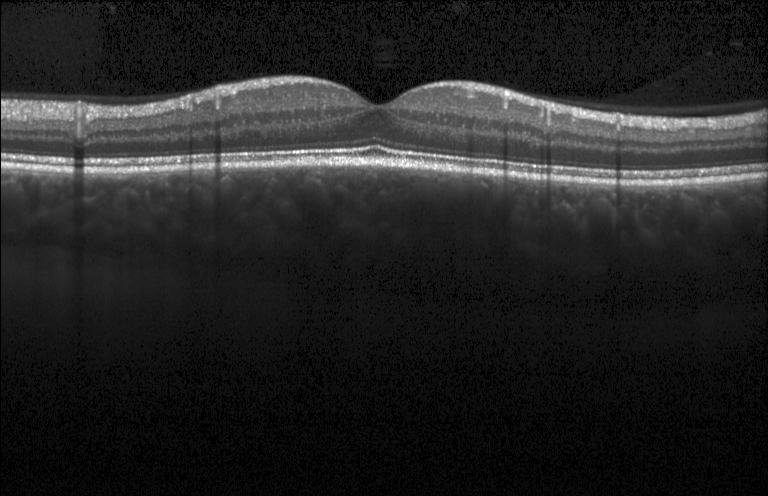

Optical coherence tomography B-scan · instrument: Heidelberg Spectralis · through the macula. Macular OCT: no choroidal neovascularization, diabetic macular edema, or drusen.